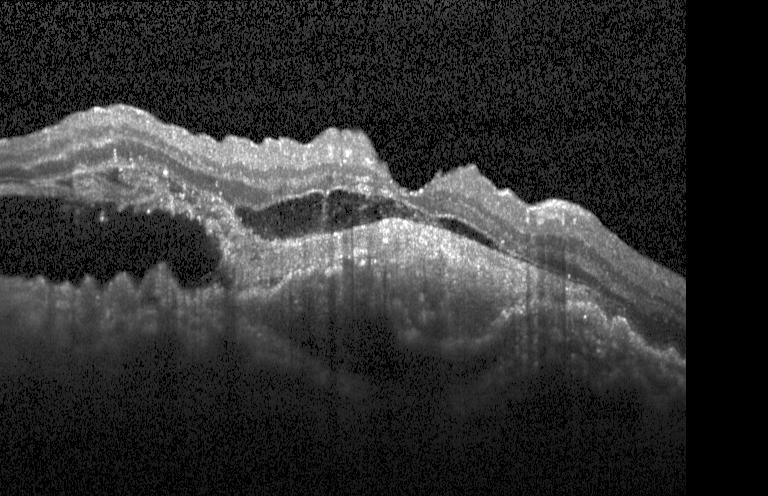 Optical coherence tomography scan. Heidelberg Spectralis OCT system. Macular scan. Spectral-domain optical coherence tomography
The scan shows CNV.